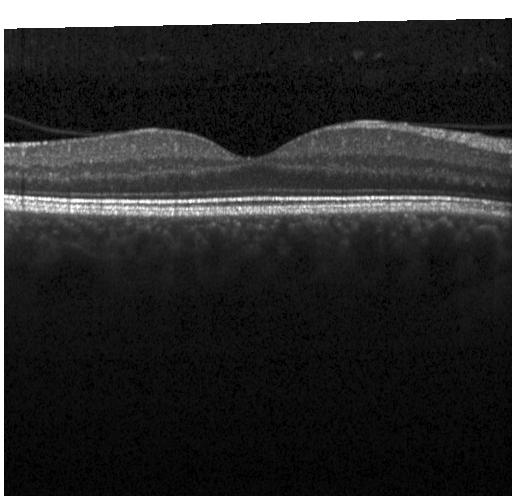
Macular scan · retinal OCT B-scan · Heidelberg Spectralis.
Finding: neither choroidal neovascularization, diabetic macular edema, nor drusen.